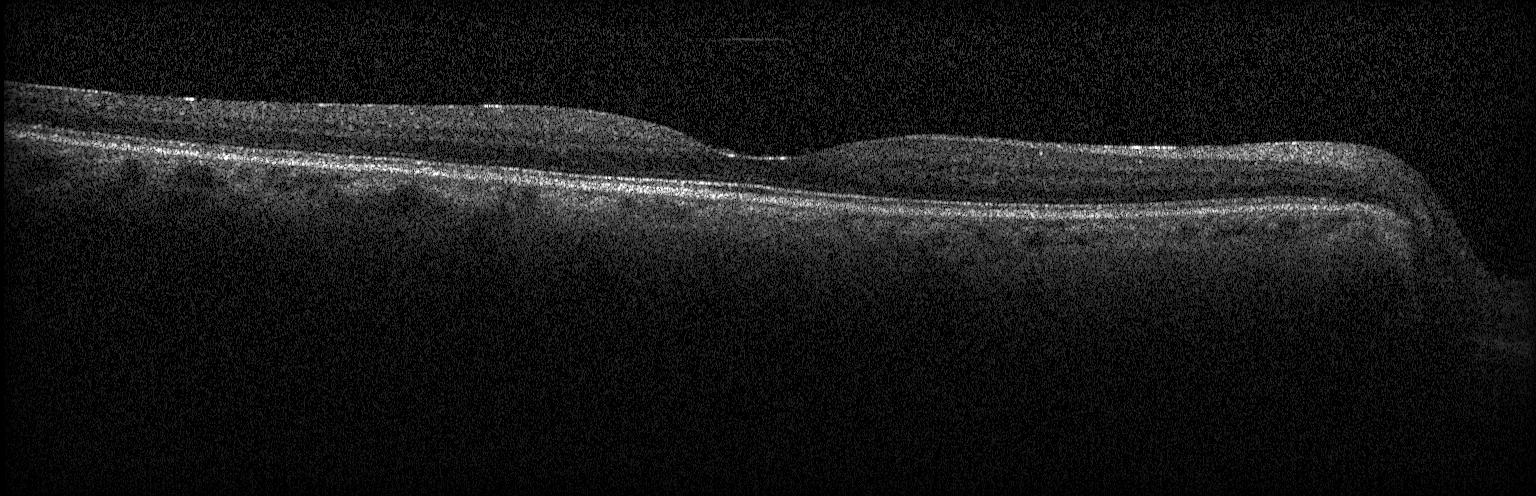 The scan shows no choroidal neovascularization, no diabetic macular edema, and no drusen.